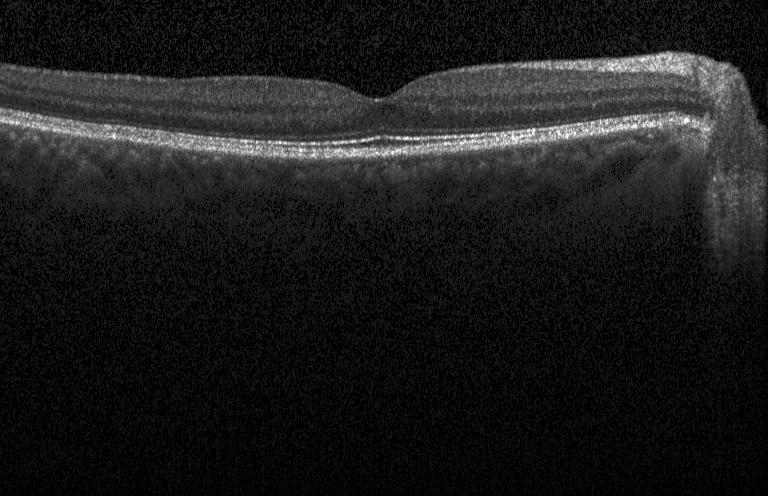

Fovea-centered, Heidelberg Spectralis OCT system, spectral-domain optical coherence tomography, optical coherence tomography B-scan.
Finding: no CNV, DME, or drusen.